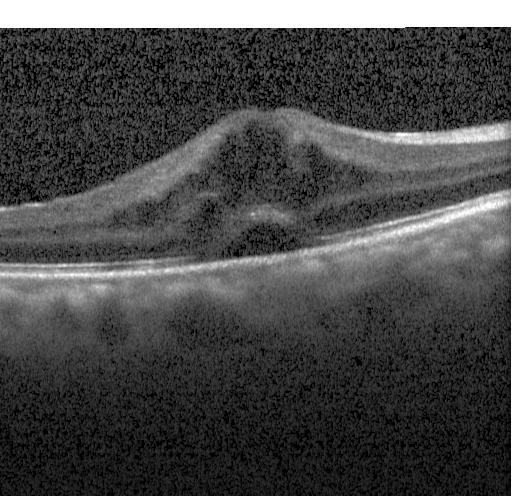
OCT line scan · SD-OCT · through the macula
Impression: diabetic macular edema.